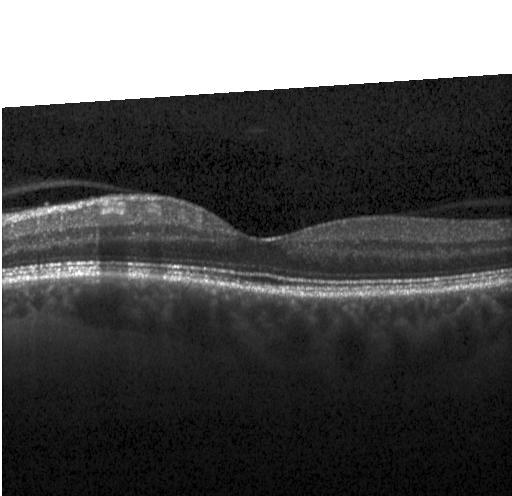

Finding: neither choroidal neovascularization, diabetic macular edema, nor drusen.